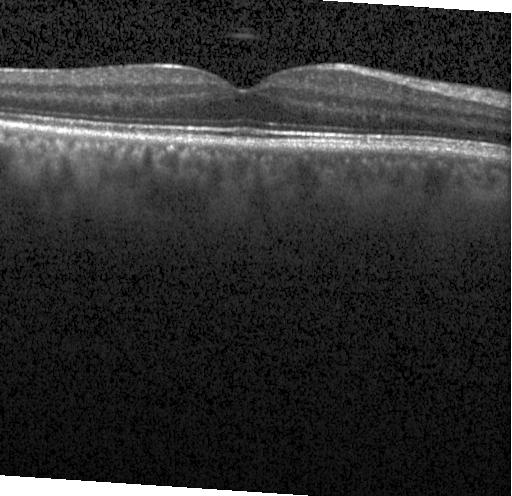 SD-OCT; optical coherence tomography scan
Diagnosis: no CNV, DME, or drusen.